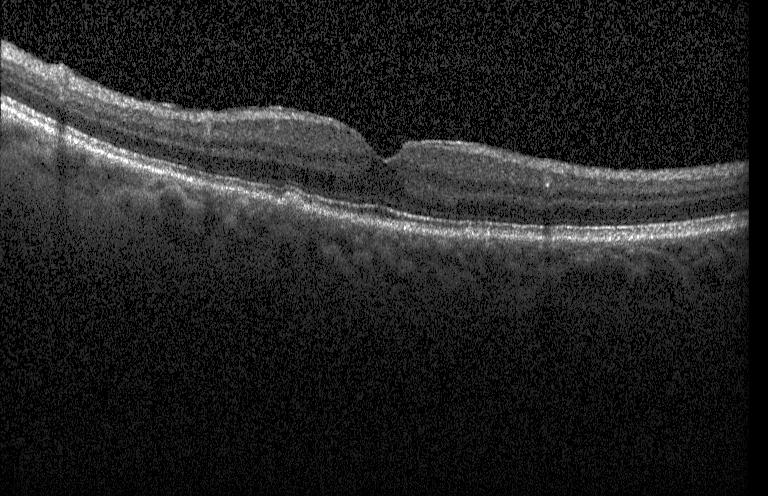 Assessment: sub-RPE drusenoid deposits.